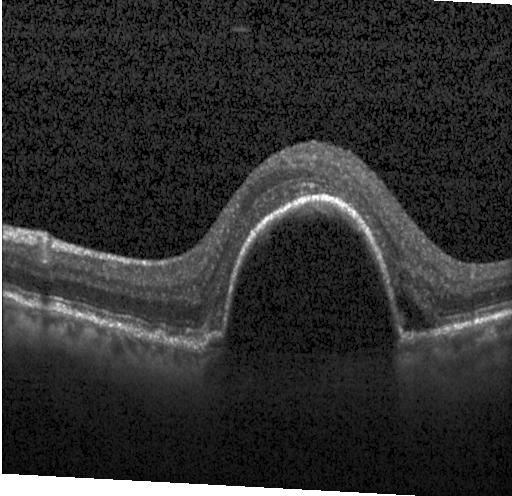

Assessment: a choroidal neovascular membrane.